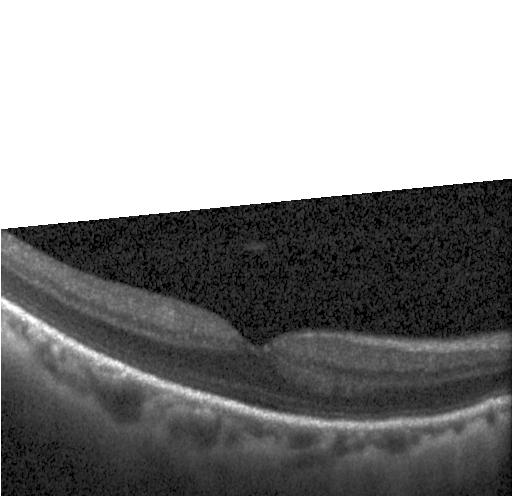 OCT finding: no CNV, DME, or drusen.